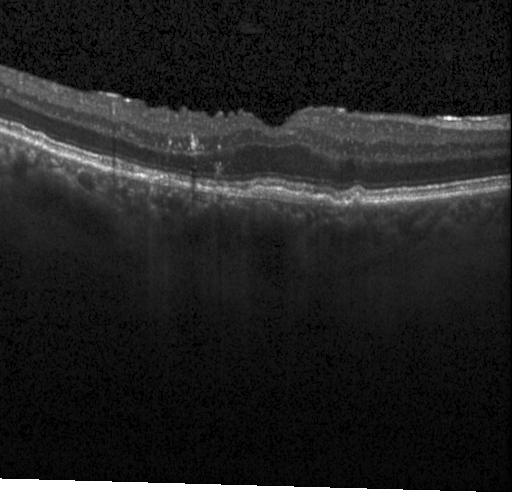

Retinal OCT cross-section. Horizontal scan through the fovea. Acquired on a Heidelberg Spectralis. Spectral-domain OCT.
Diagnosis: choroidal neovascularization (CNV).